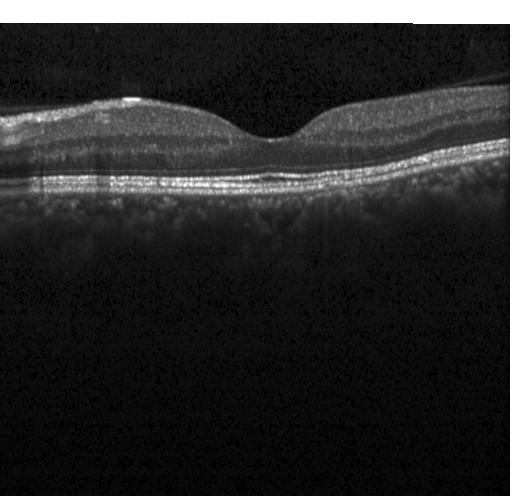

Neither CNV, DME, nor drusen.